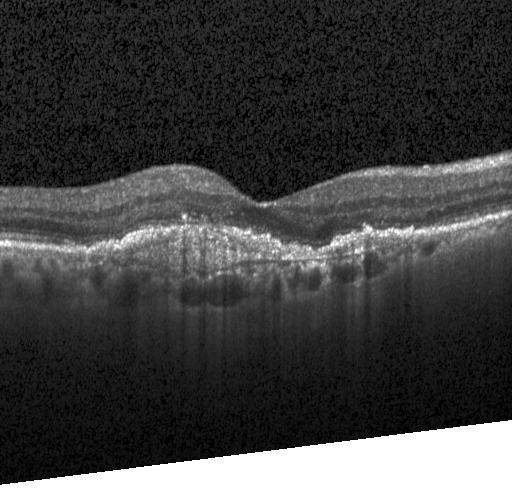
Dx: choroidal neovascularization (CNV).